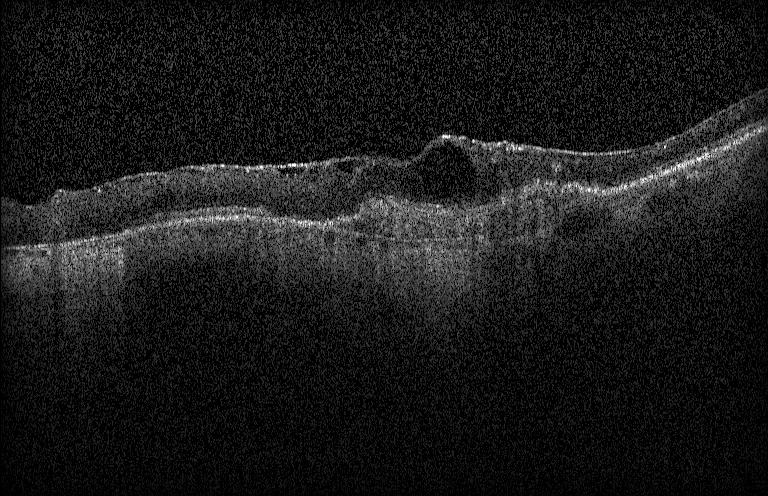
SD-OCT; retinal OCT cross-section. Macular OCT: a choroidal neovascular membrane.